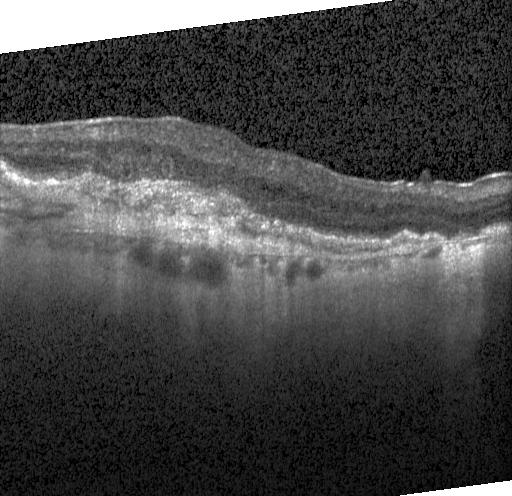

Retinal OCT cross-section, centered on the fovea, Heidelberg Spectralis OCT system.
Assessment: a choroidal neovascular membrane.